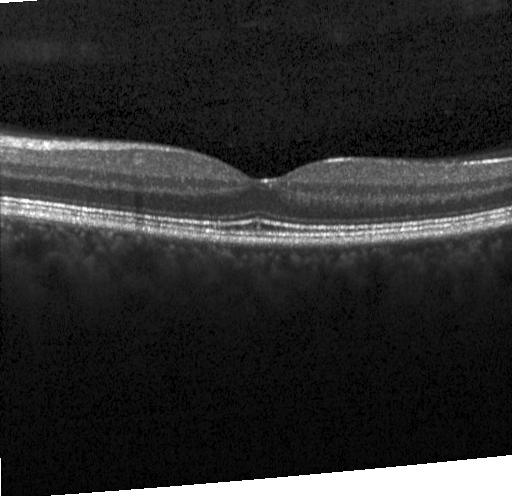 Acquired on a Heidelberg Spectralis; OCT B-scan; through the macula; spectral-domain optical coherence tomography. This B-scan demonstrates no choroidal neovascularization, no diabetic macular edema, and no drusen.